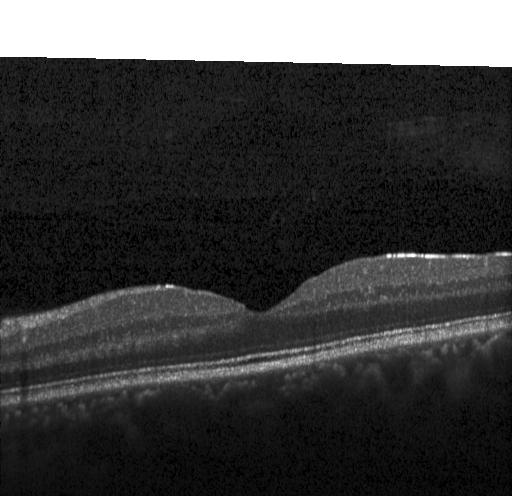
Through the macula, retinal OCT cross-section, acquired on a Heidelberg Spectralis, spectral-domain OCT — Finding: no CNV, no DME, and no drusen.